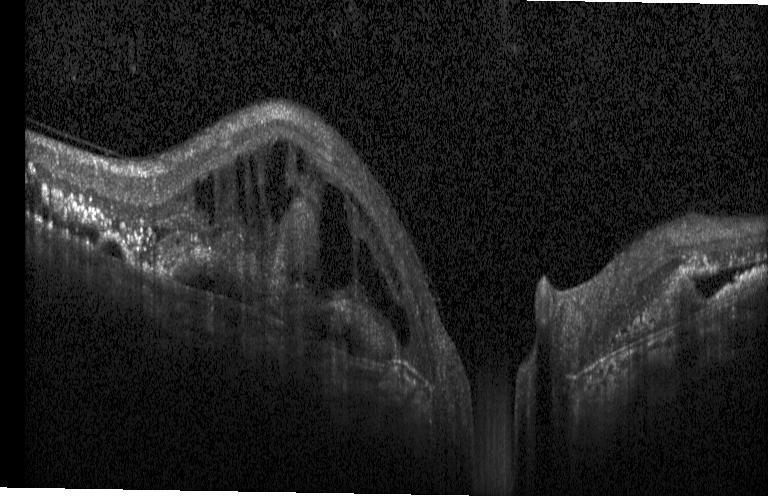

Optical coherence tomography scan — Macular OCT: a choroidal neovascular membrane.